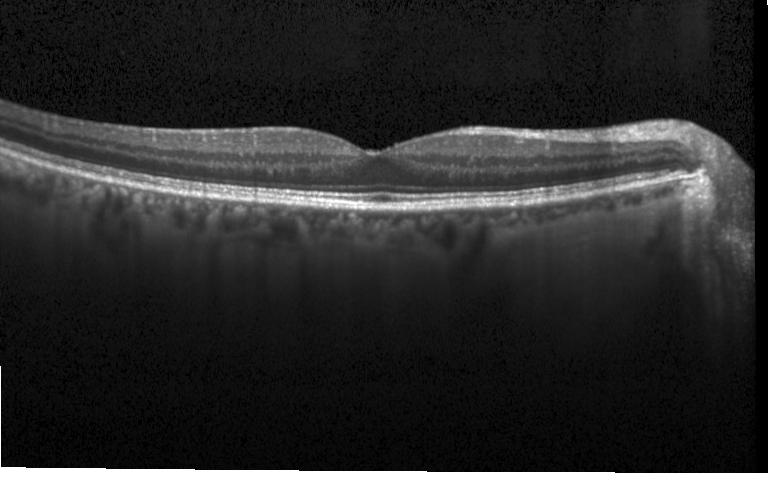
Finding: neither choroidal neovascularization, diabetic macular edema, nor drusen.